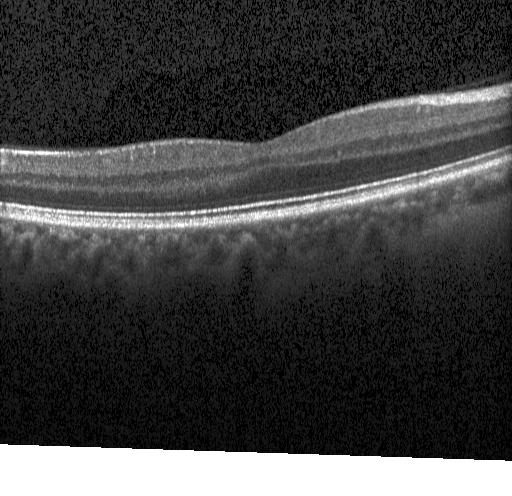
Macular OCT demonstrating neither choroidal neovascularization, diabetic macular edema, nor drusen.